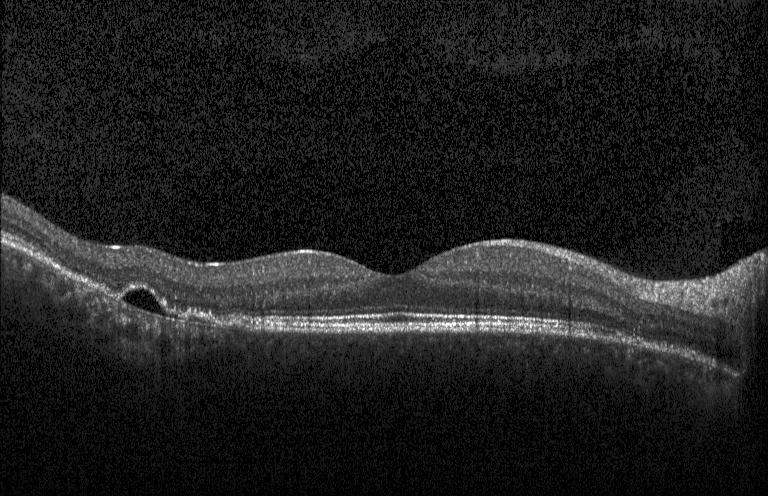 A choroidal neovascular membrane.